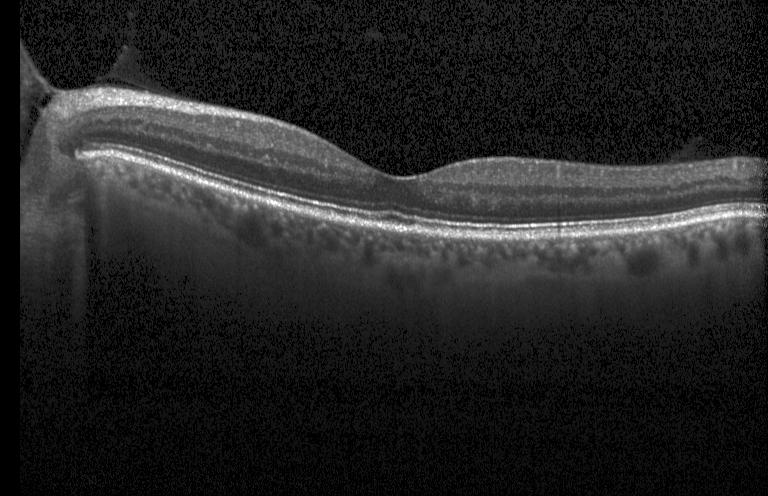
Centered on the fovea. Spectral-domain optical coherence tomography. Retinal OCT cross-section. Macular OCT: no CNV, no DME, and no drusen.